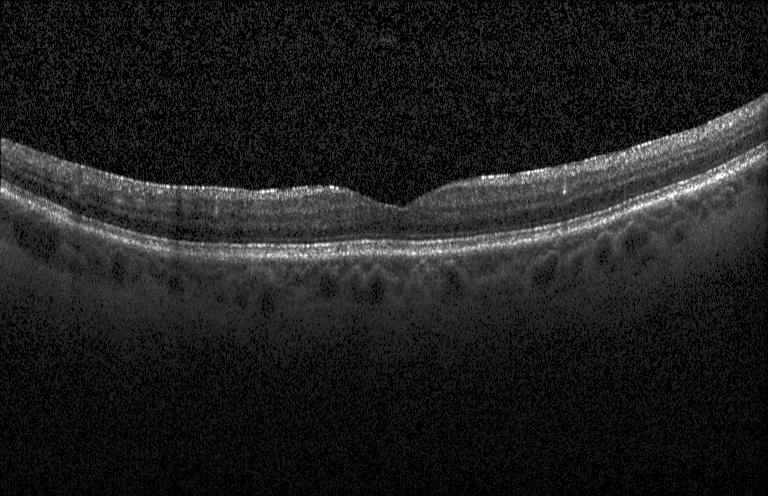

Macular OCT: no evidence of choroidal neovascularization, diabetic macular edema, or drusen.